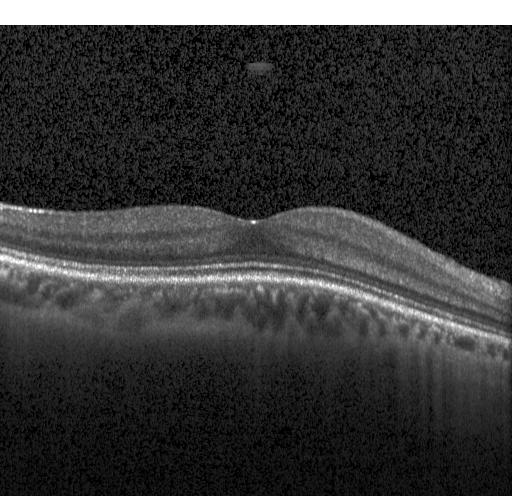

Spectral-domain OCT; through the macula; Heidelberg Spectralis; retinal OCT B-scan — No choroidal neovascularization, diabetic macular edema, or drusen.